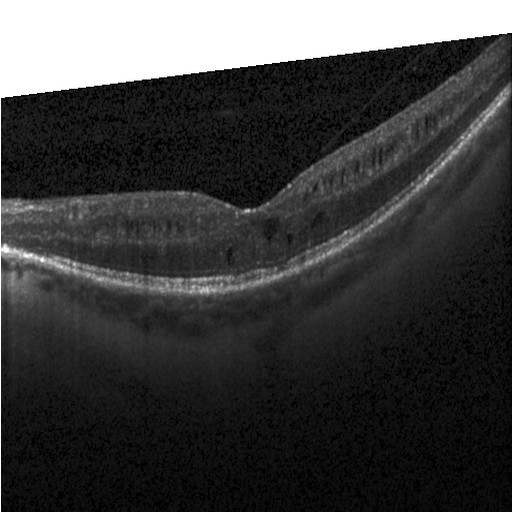 Macular OCT: diabetic macular edema.